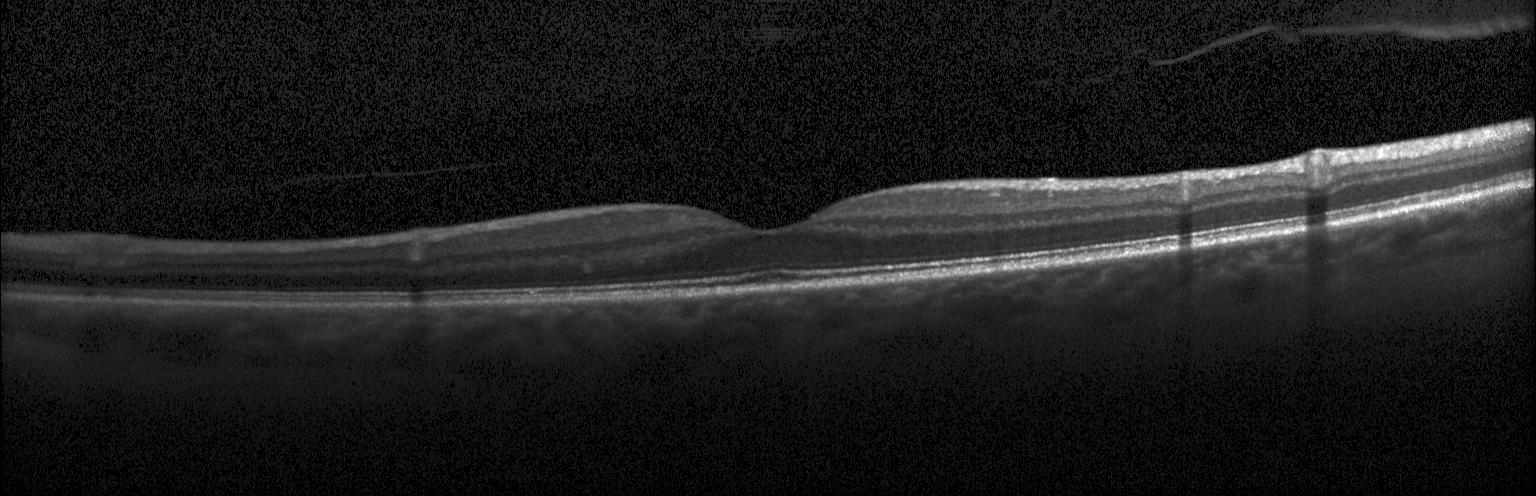

OCT finding: no choroidal neovascularization, diabetic macular edema, or drusen.